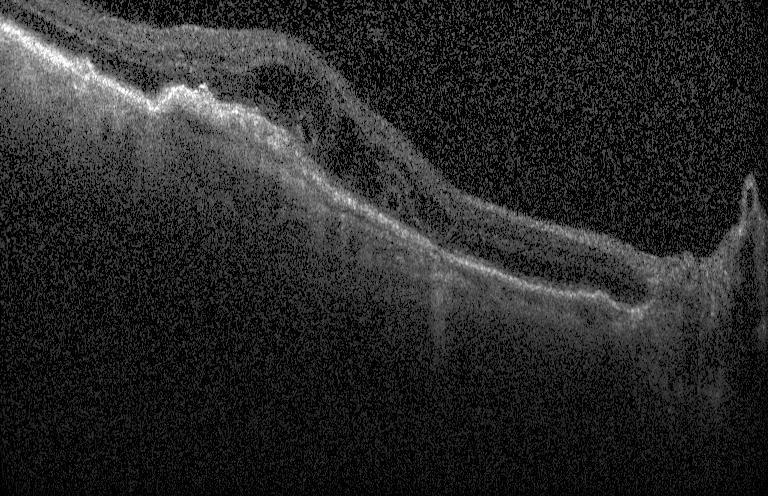
OCT B-scan, Heidelberg Spectralis OCT system
OCT finding: a choroidal neovascular membrane.